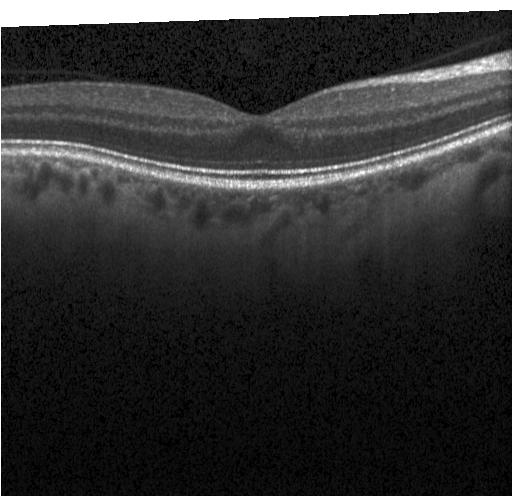

Horizontal scan through the fovea. Retinal OCT B-scan. Spectral-domain OCT. Acquired on a Heidelberg Spectralis — Impression: neither choroidal neovascularization, diabetic macular edema, nor drusen.